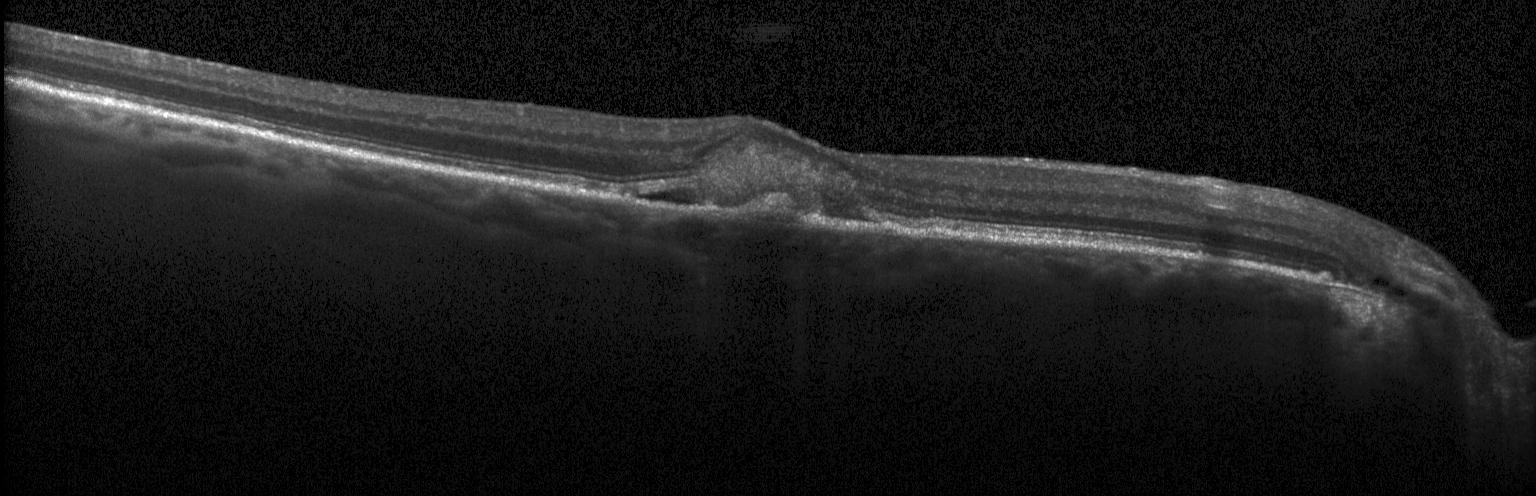

Spectral-domain OCT. Heidelberg Spectralis. Optical coherence tomography scan. Macular scan.
Impression: a choroidal neovascular membrane.